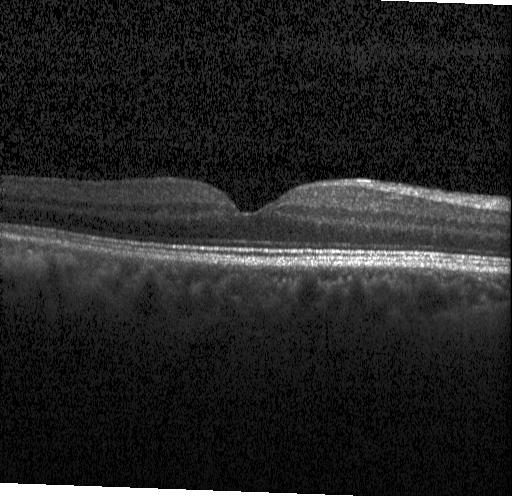
Diagnosis: neither CNV, DME, nor drusen.